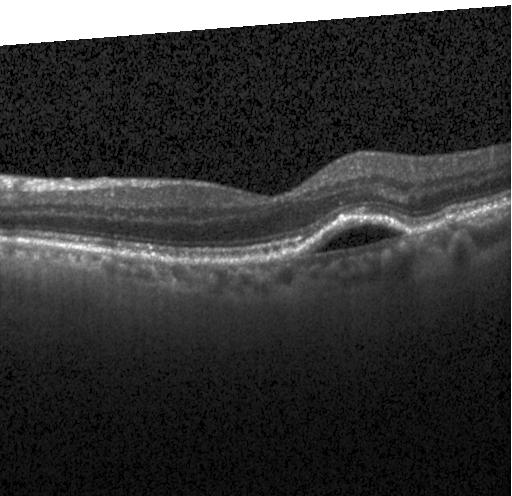
Macular OCT: a choroidal neovascular membrane.